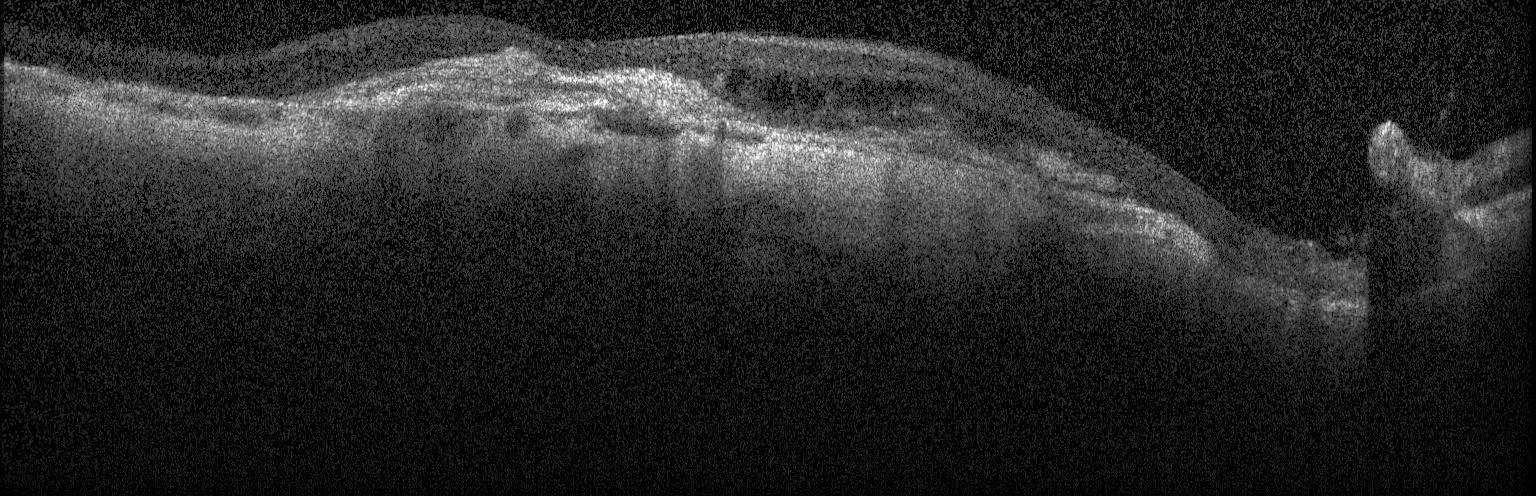 Assessment: a choroidal neovascular membrane.